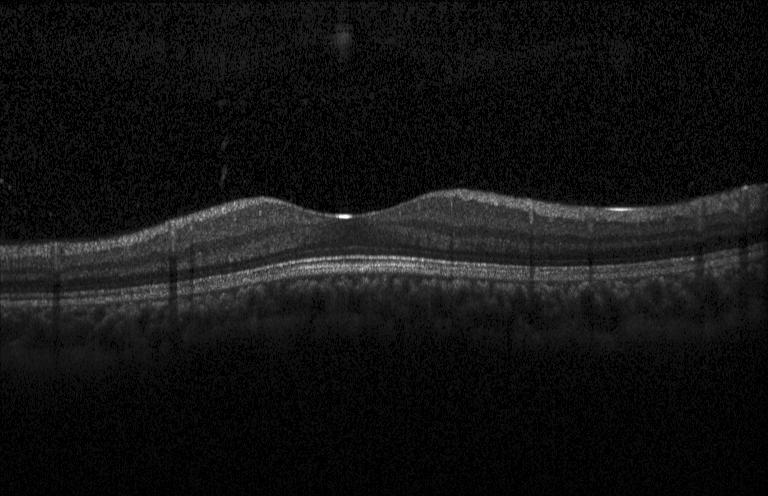
Spectral-domain OCT B-scan: neither choroidal neovascularization, diabetic macular edema, nor drusen.